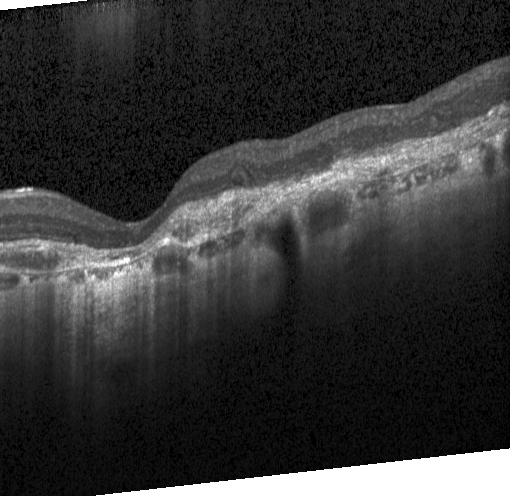
Impression: CNV.